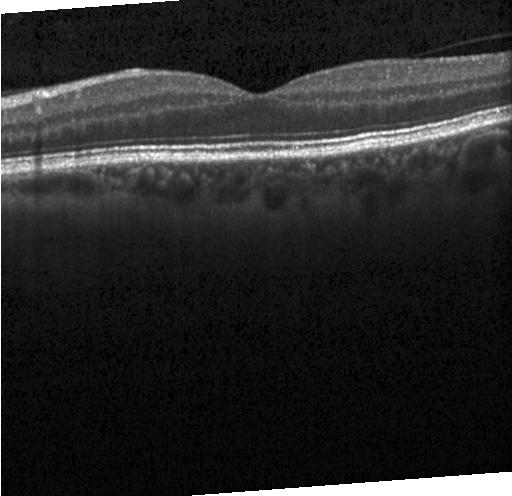 Dx: no choroidal neovascularization, no diabetic macular edema, and no drusen.